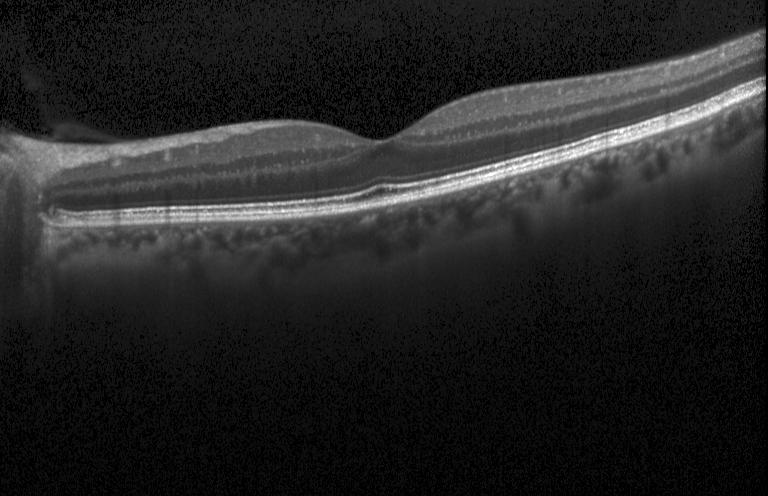 Retinal OCT cross-section · spectral-domain OCT · fovea-centered
Diagnosis: no choroidal neovascularization, no diabetic macular edema, and no drusen.